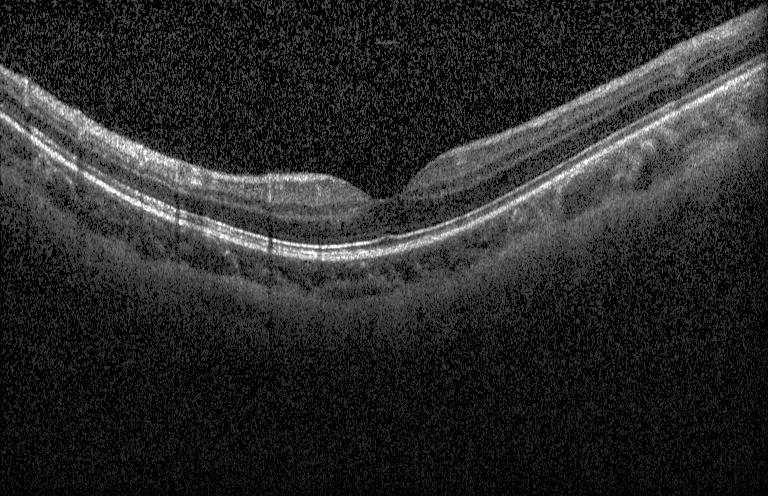
Through the macula; SD-OCT; Heidelberg Spectralis; OCT B-scan
Impression: no CNV, no DME, and no drusen.